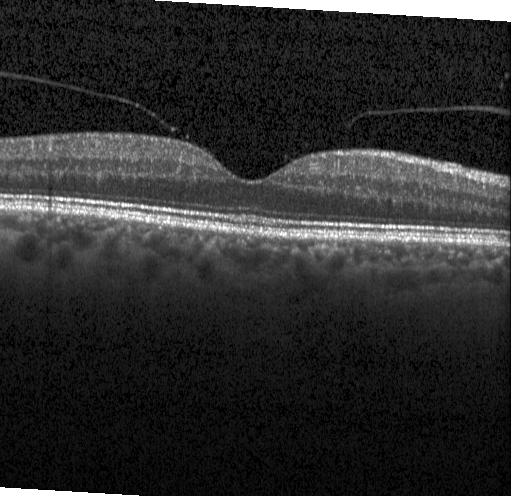

Optical coherence tomography B-scan.
Finding: no choroidal neovascularization, no diabetic macular edema, and no drusen.